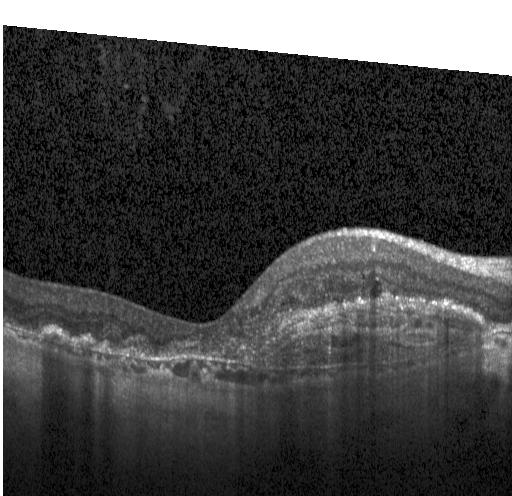
Retinal OCT cross-section showing choroidal neovascularization.